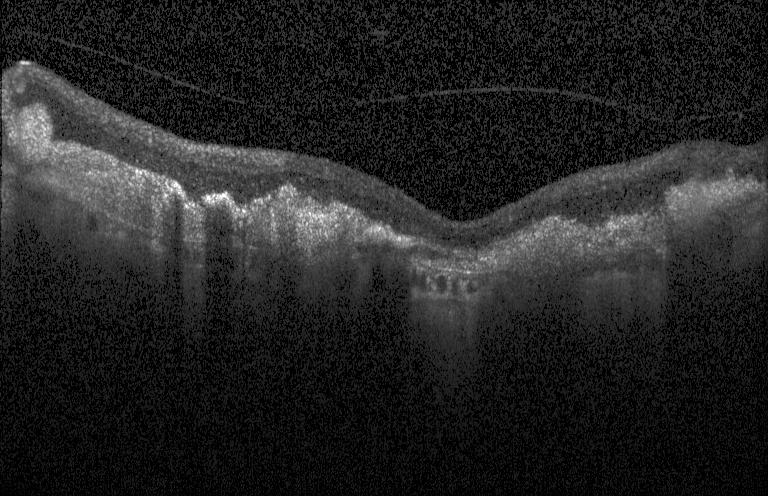
Instrument: Heidelberg Spectralis, centered on the fovea, optical coherence tomography scan, SD-OCT.
Diagnosis: a choroidal neovascular membrane.